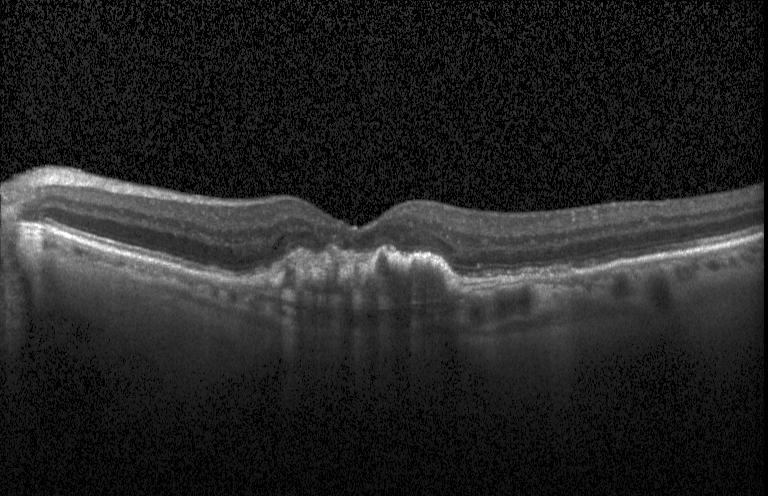

Fovea-centered. Spectral-domain OCT. OCT B-scan. Dx: a choroidal neovascular membrane.